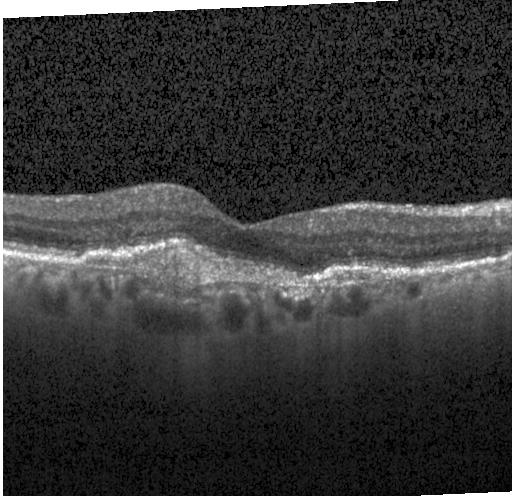
Spectral-domain OCT; fovea-centered; optical coherence tomography scan; instrument: Heidelberg Spectralis.
Diagnosis: choroidal neovascularization.